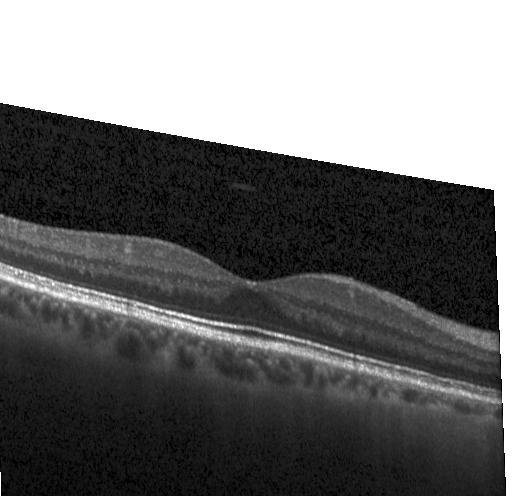

OCT B-scan · centered on the fovea. Impression: no choroidal neovascularization, diabetic macular edema, or drusen.